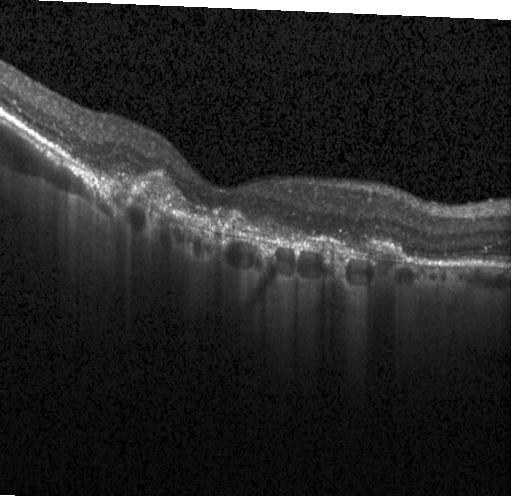
OCT scan showing a choroidal neovascular membrane.